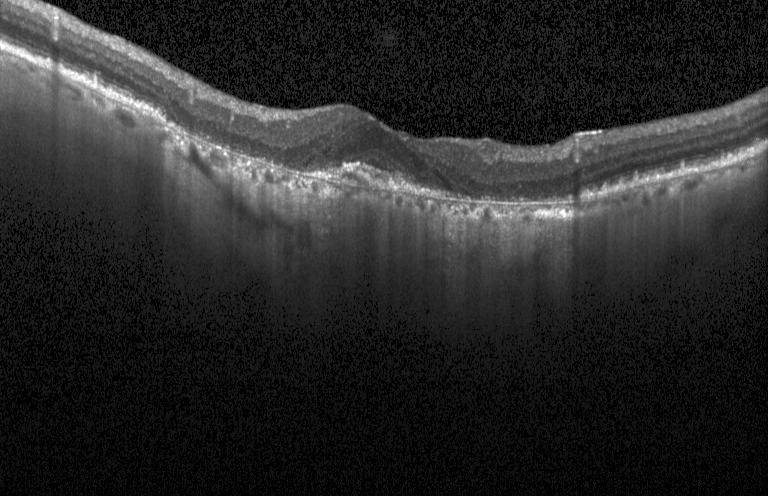
OCT line scan
CNV.